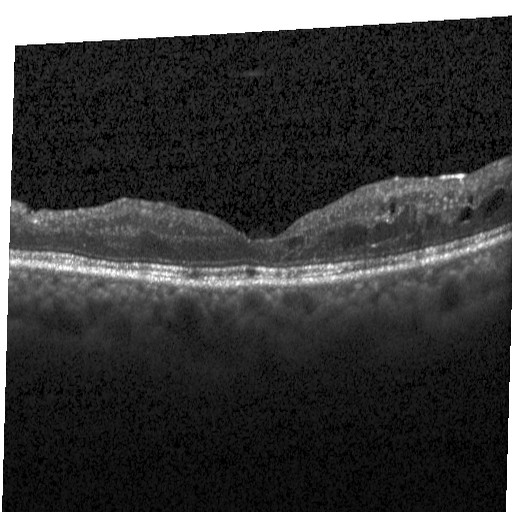

OCT line scan. Diagnosis: diabetic macular edema.